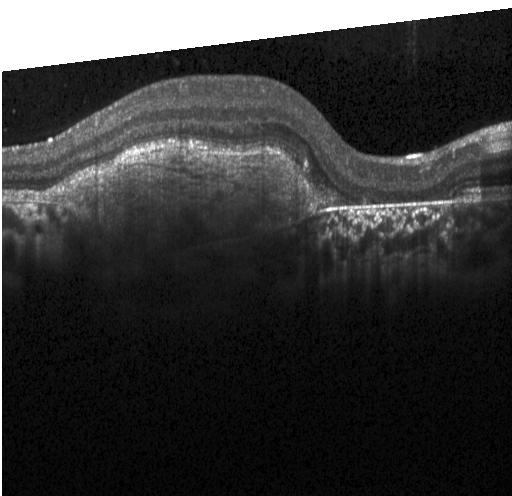 Diagnosis: CNV.